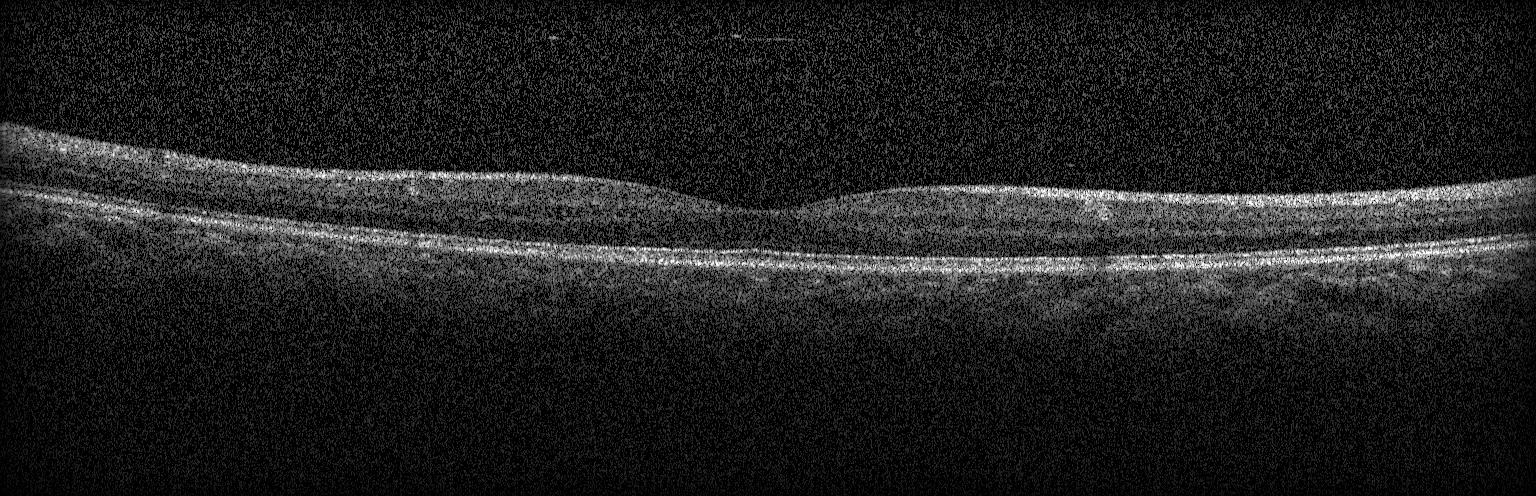

Optical coherence tomography B-scan · fovea-centered
Diagnosis: no evidence of CNV, DME, or drusen.